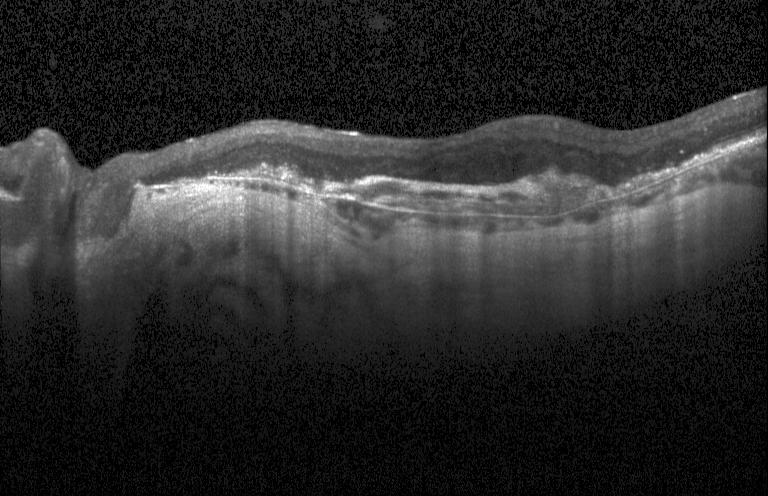 Optical coherence tomography B-scan — This B-scan demonstrates a choroidal neovascular membrane.